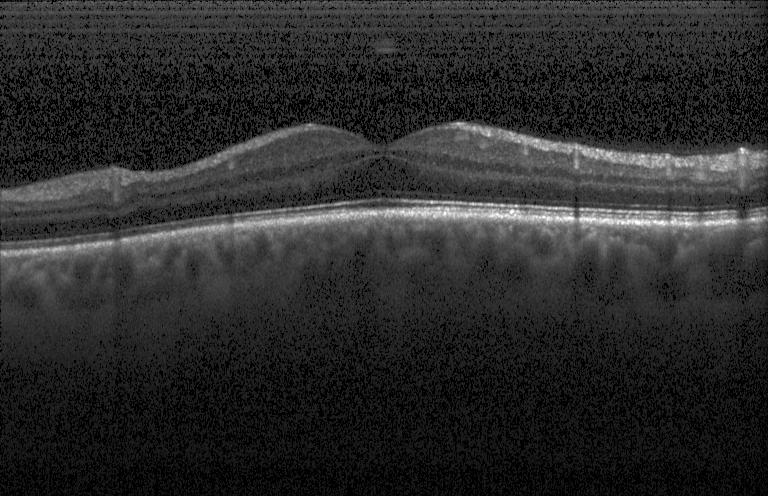
OCT scan showing neither choroidal neovascularization, diabetic macular edema, nor drusen.